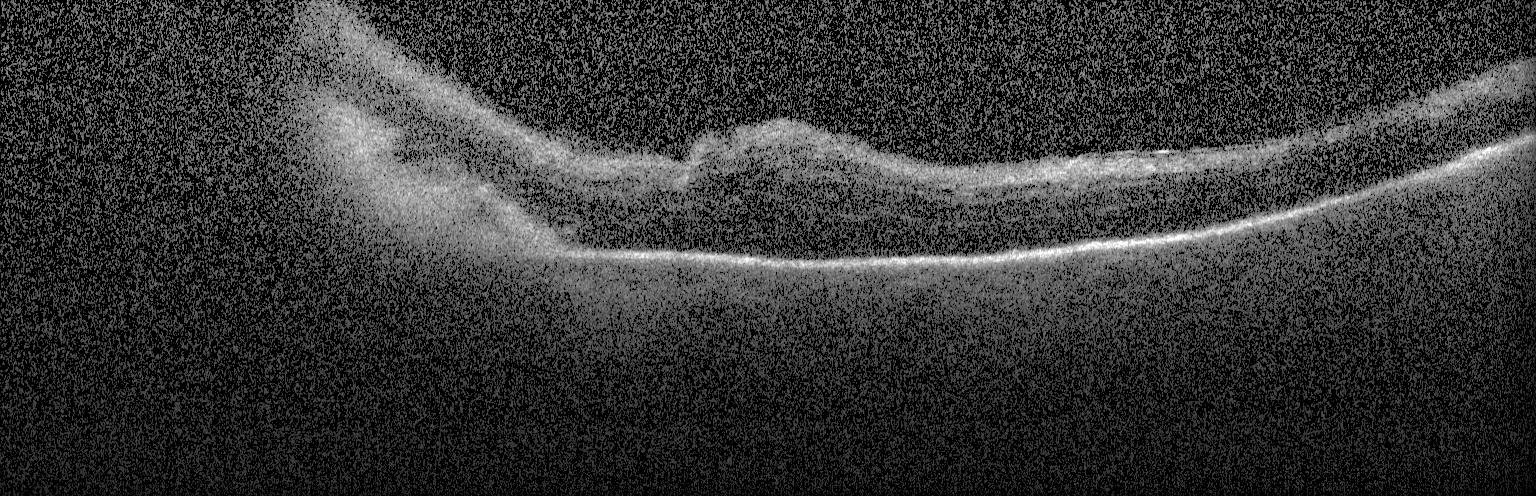
Diagnosis: diabetic macular edema.